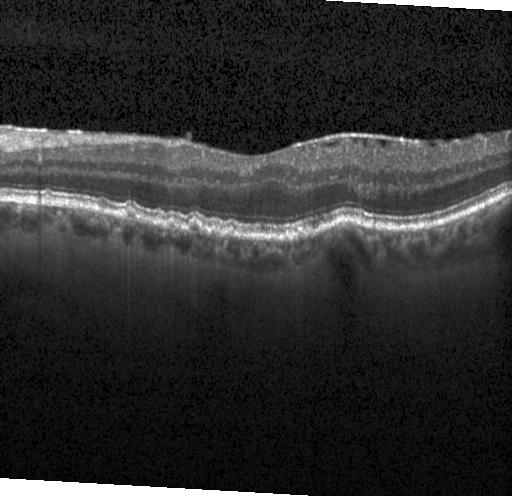

Retinal OCT B-scan.
The scan shows multiple drusen.